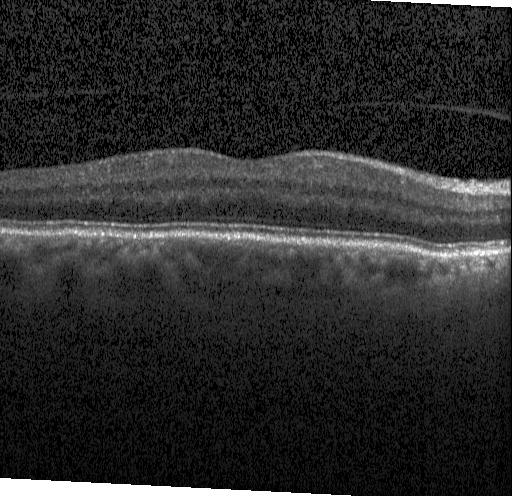 OCT line scan. Through the macula.
Finding: neither choroidal neovascularization, diabetic macular edema, nor drusen.